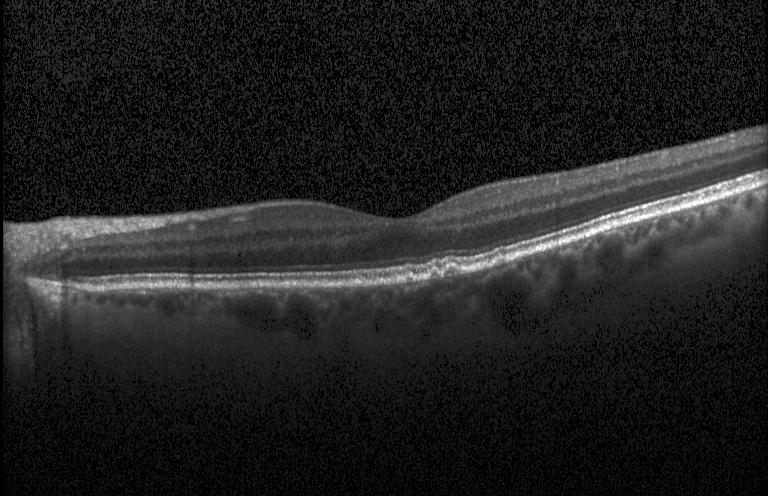

SD-OCT. OCT B-scan. Through the macula. Acquired on a Heidelberg Spectralis — The scan shows multiple drusen.